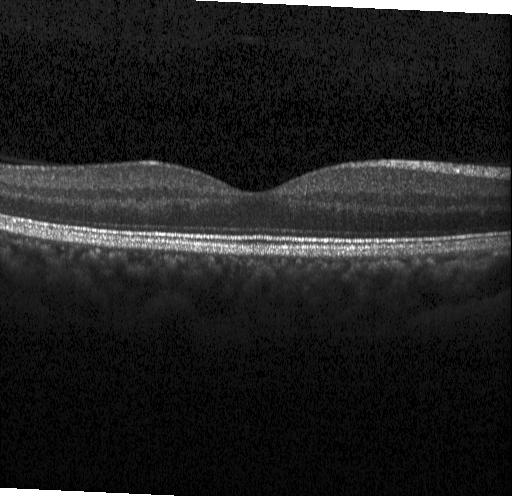
Retinal OCT B-scan. OCT finding: no choroidal neovascularization, no diabetic macular edema, and no drusen.